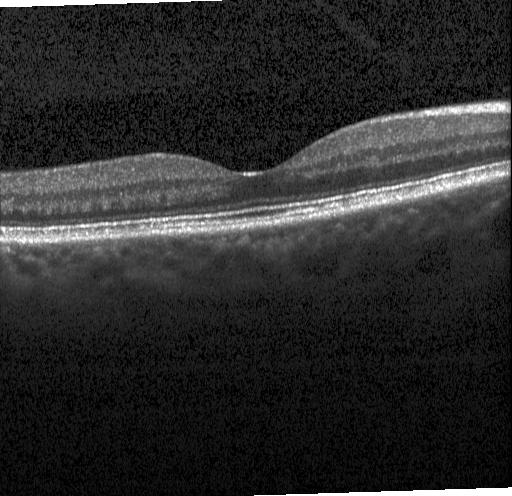

Optical coherence tomography scan. Fovea-centered. Diagnosis: no evidence of choroidal neovascularization, diabetic macular edema, or drusen.